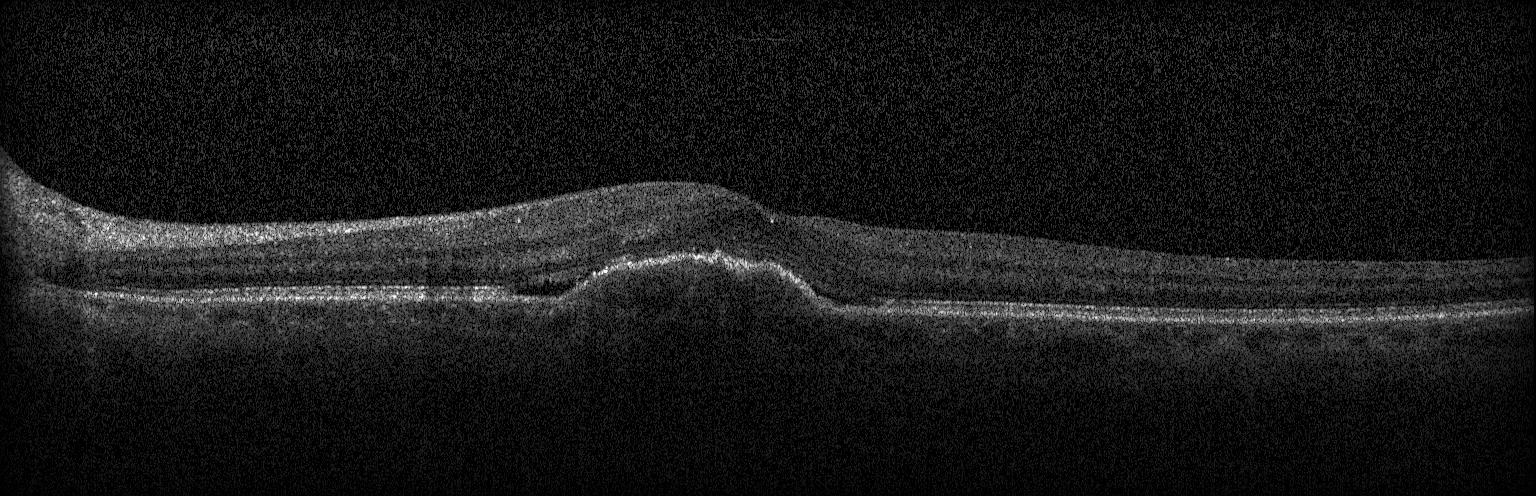 Macular OCT demonstrating choroidal neovascularization (CNV).